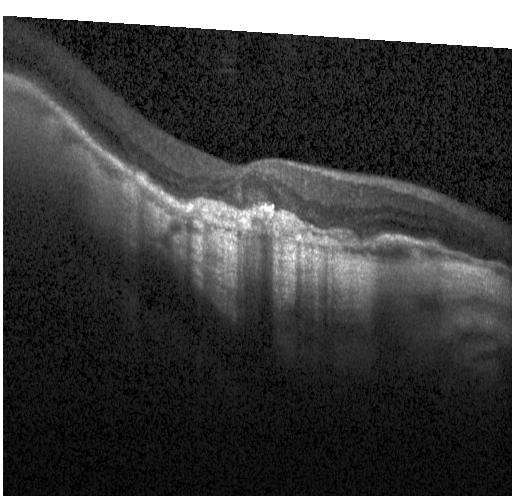
Optical coherence tomography B-scan
Impression: a choroidal neovascular membrane.